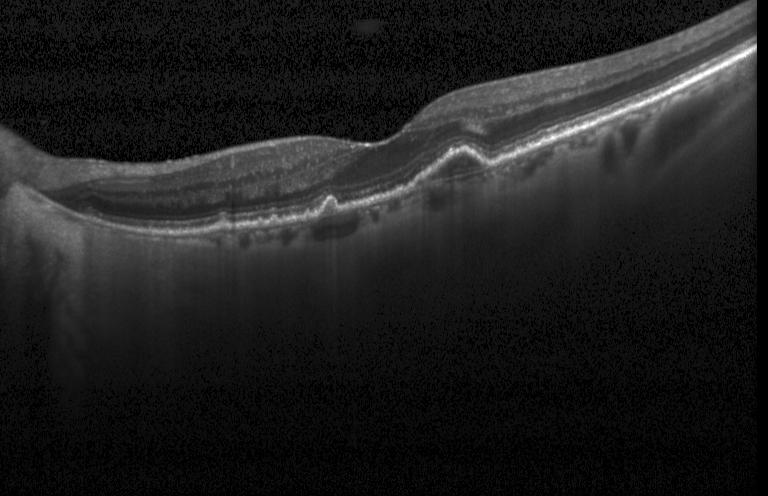 Assessment: choroidal neovascularization.